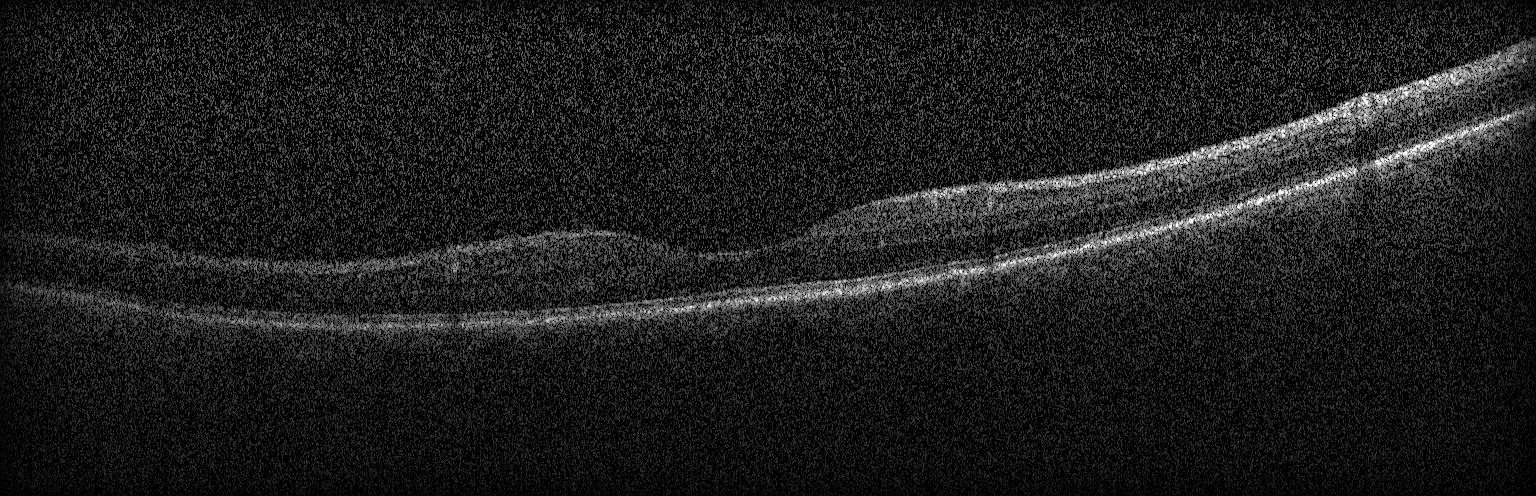 OCT B-scan · SD-OCT. The scan shows neither CNV, DME, nor drusen.